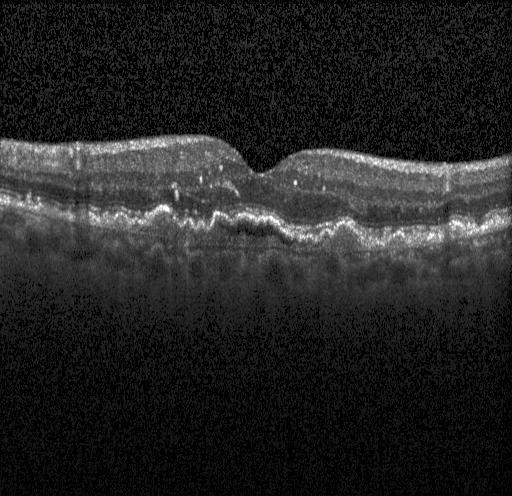

Spectral-domain OCT · macular scan · optical coherence tomography B-scan — A choroidal neovascular membrane.